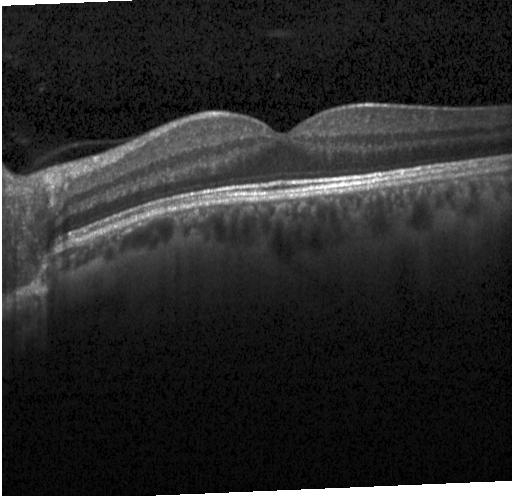
Retinal OCT cross-section · spectral-domain OCT
Finding: no choroidal neovascularization, diabetic macular edema, or drusen.